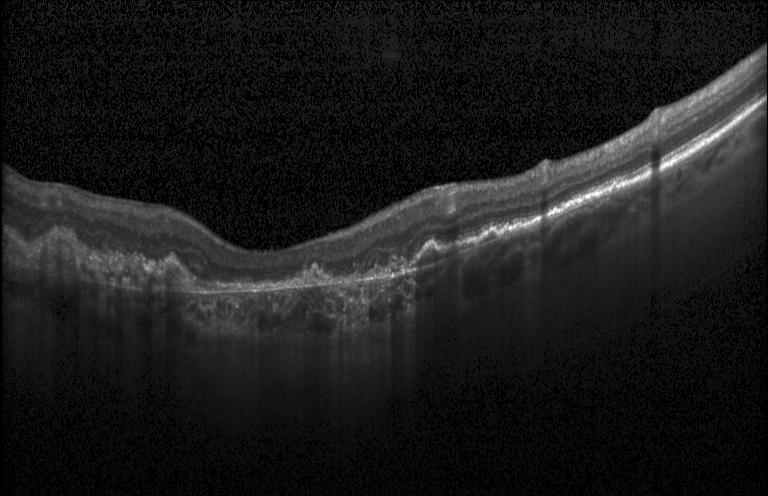 Retinal OCT B-scan.
The scan shows a choroidal neovascular membrane.